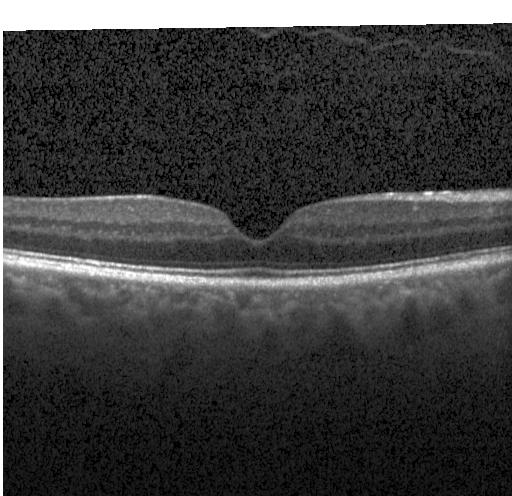
Impression: no choroidal neovascularization, diabetic macular edema, or drusen.